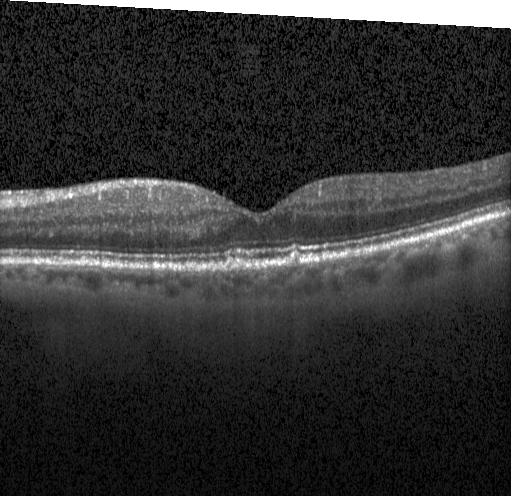

Horizontal scan through the fovea · optical coherence tomography B-scan
Finding: sub-RPE drusenoid deposits.